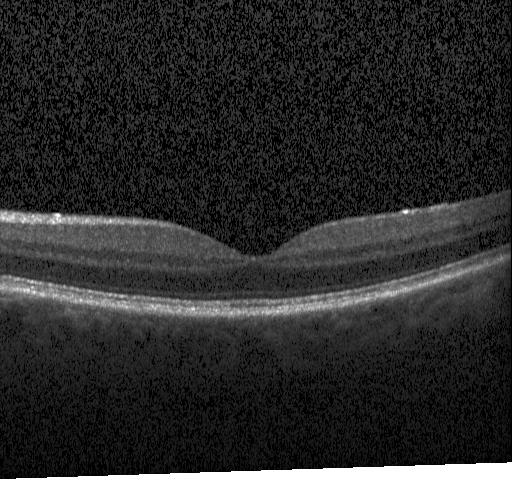
Spectral-domain OCT B-scan: no choroidal neovascularization, diabetic macular edema, or drusen.